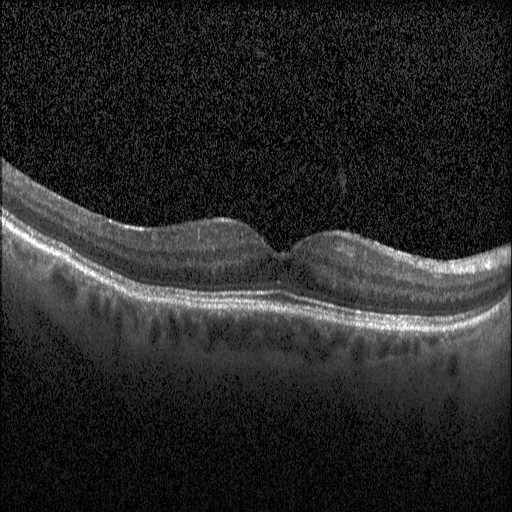

Finding: diabetic macular edema (DME).